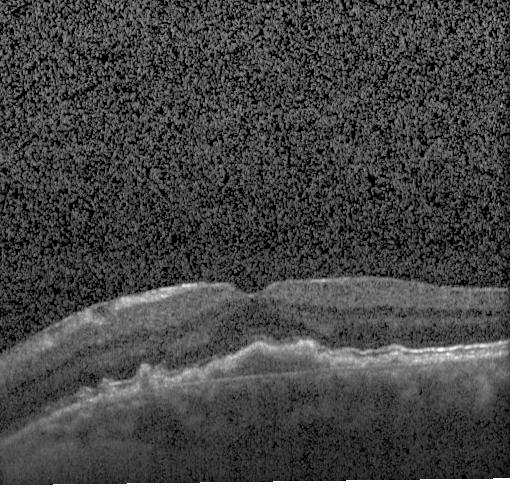 Heidelberg Spectralis OCT system, macular scan, spectral-domain OCT, OCT B-scan. The scan shows a choroidal neovascular membrane.